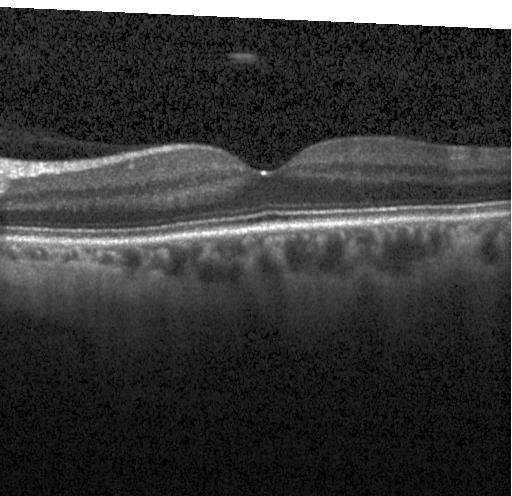

Optical coherence tomography scan; spectral-domain optical coherence tomography; instrument: Heidelberg Spectralis — Assessment: no choroidal neovascularization, no diabetic macular edema, and no drusen.